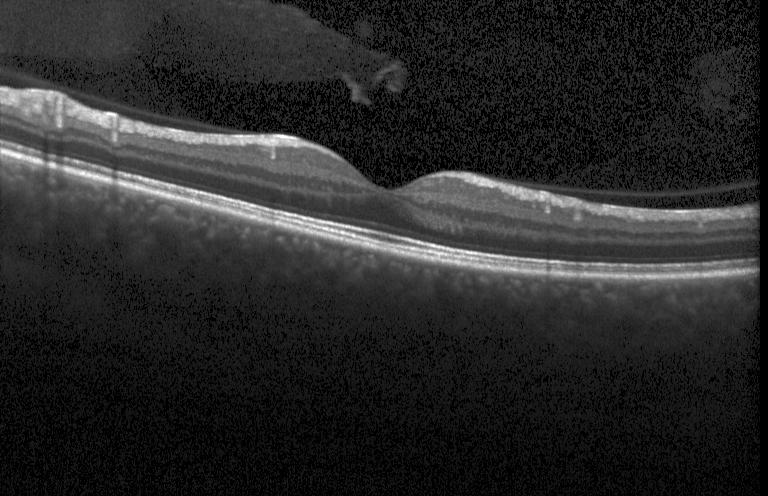 Impression: no choroidal neovascularization, diabetic macular edema, or drusen.